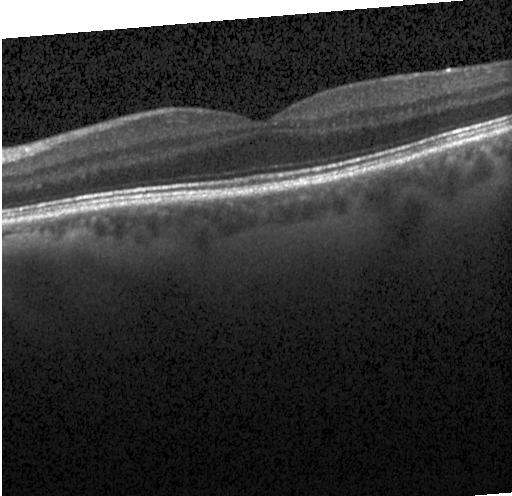 Heidelberg Spectralis OCT system; optical coherence tomography B-scan
This B-scan demonstrates no choroidal neovascularization, diabetic macular edema, or drusen.